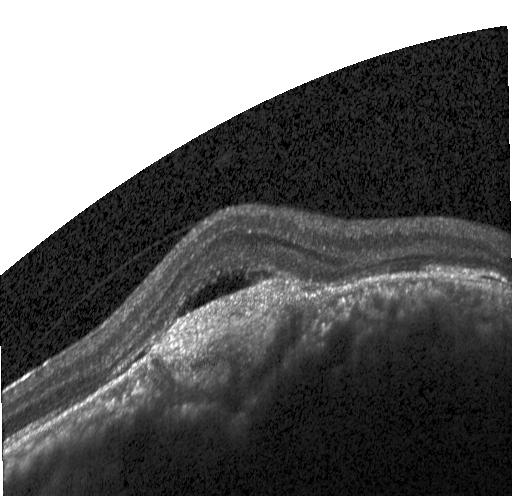 Optical coherence tomography scan. The scan shows choroidal neovascularization (CNV).